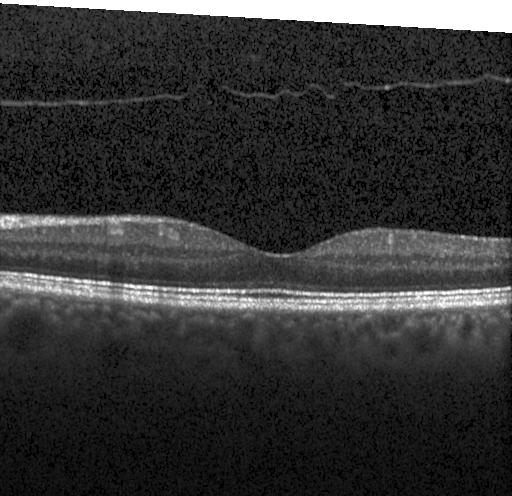
OCT line scan, instrument: Heidelberg Spectralis, spectral-domain OCT, fovea-centered. No choroidal neovascularization, no diabetic macular edema, and no drusen.